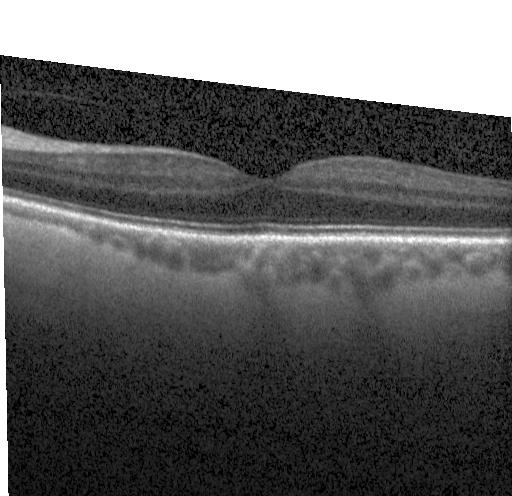

Finding: no choroidal neovascularization, no diabetic macular edema, and no drusen.